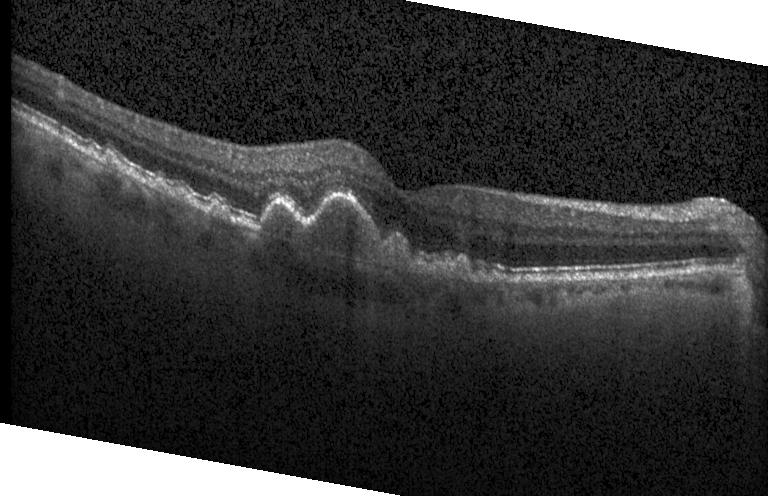 Spectral-domain OCT B-scan: a choroidal neovascular membrane.